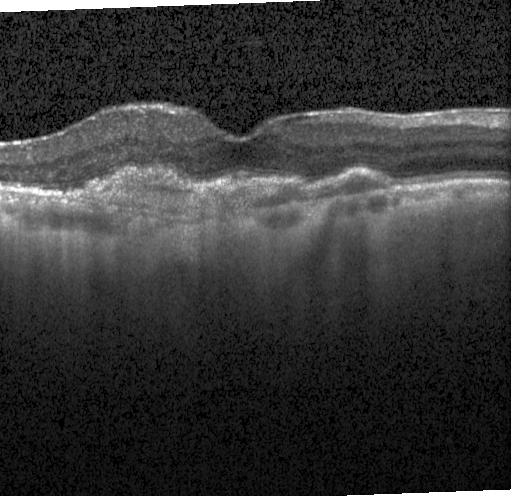 Retinal OCT B-scan
Diagnosis: choroidal neovascularization (CNV).